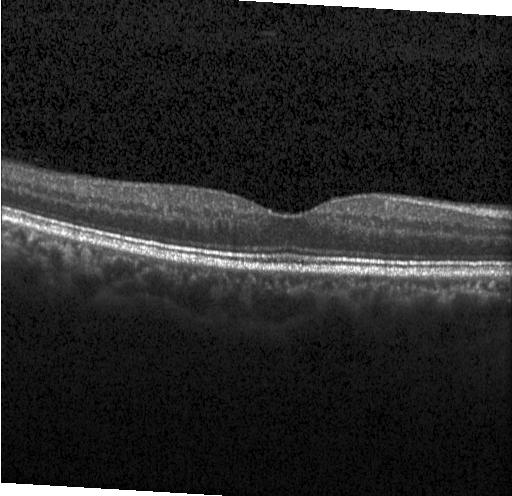
Assessment: no CNV, DME, or drusen.